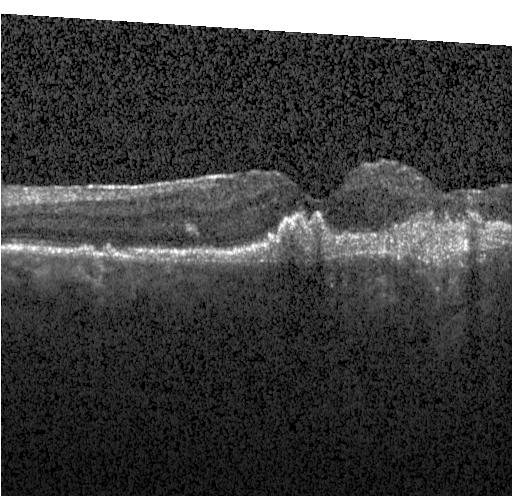

A choroidal neovascular membrane.